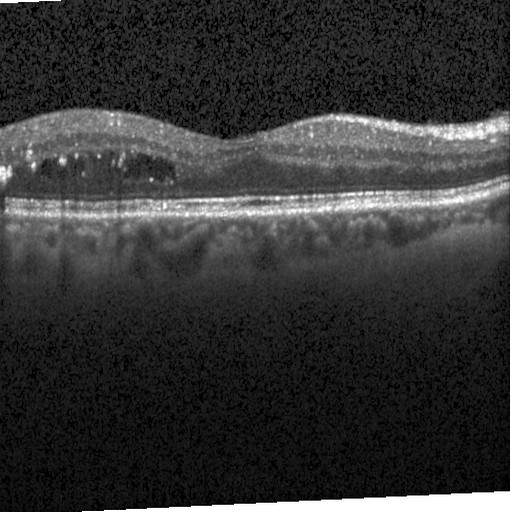

Impression: DME.